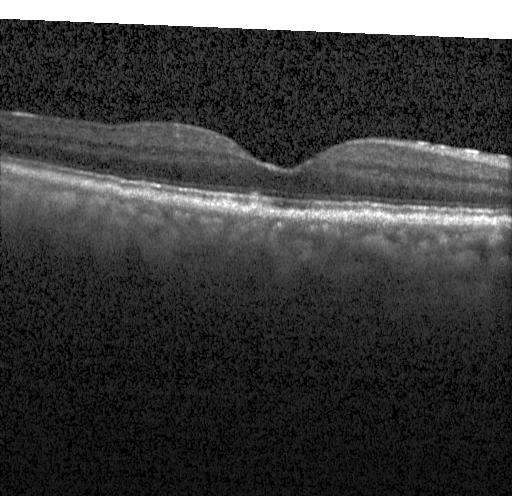
Instrument: Heidelberg Spectralis, horizontal scan through the fovea, OCT line scan, SD-OCT. This B-scan demonstrates drusen.